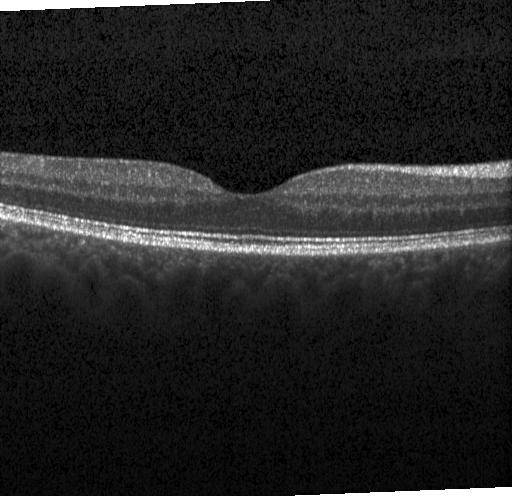

Horizontal scan through the fovea, spectral-domain optical coherence tomography, retinal OCT cross-section.
Diagnosis: no evidence of choroidal neovascularization, diabetic macular edema, or drusen.